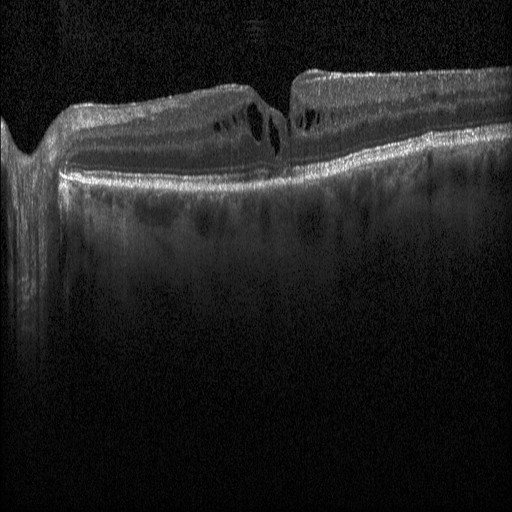

This B-scan demonstrates DME.